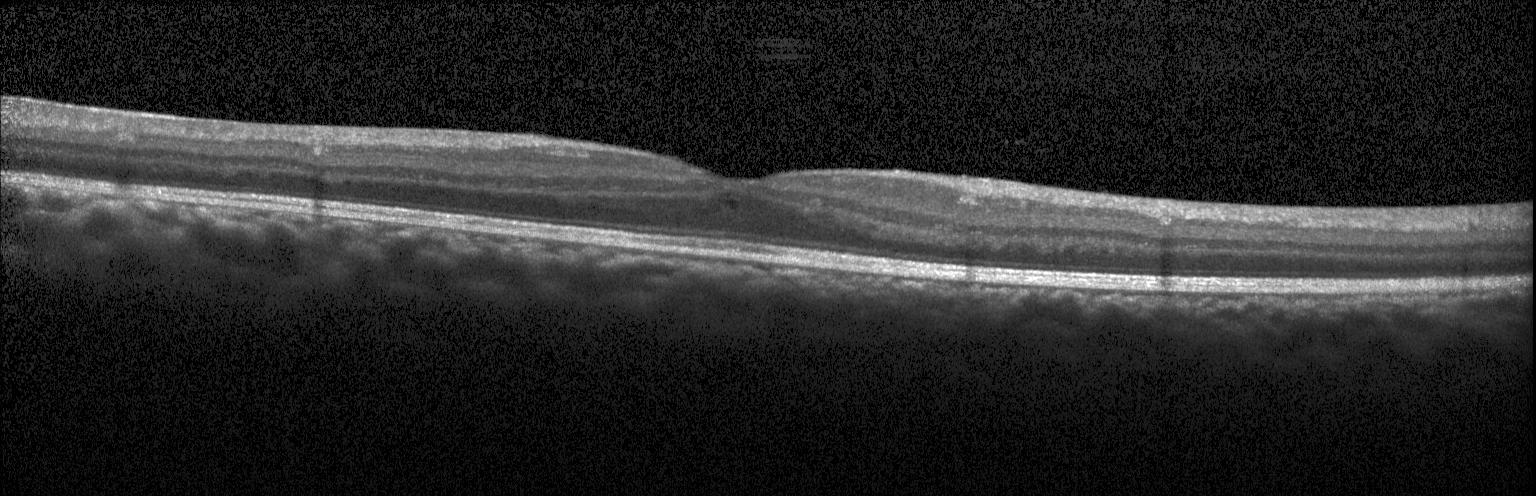

Diagnosis: DME.